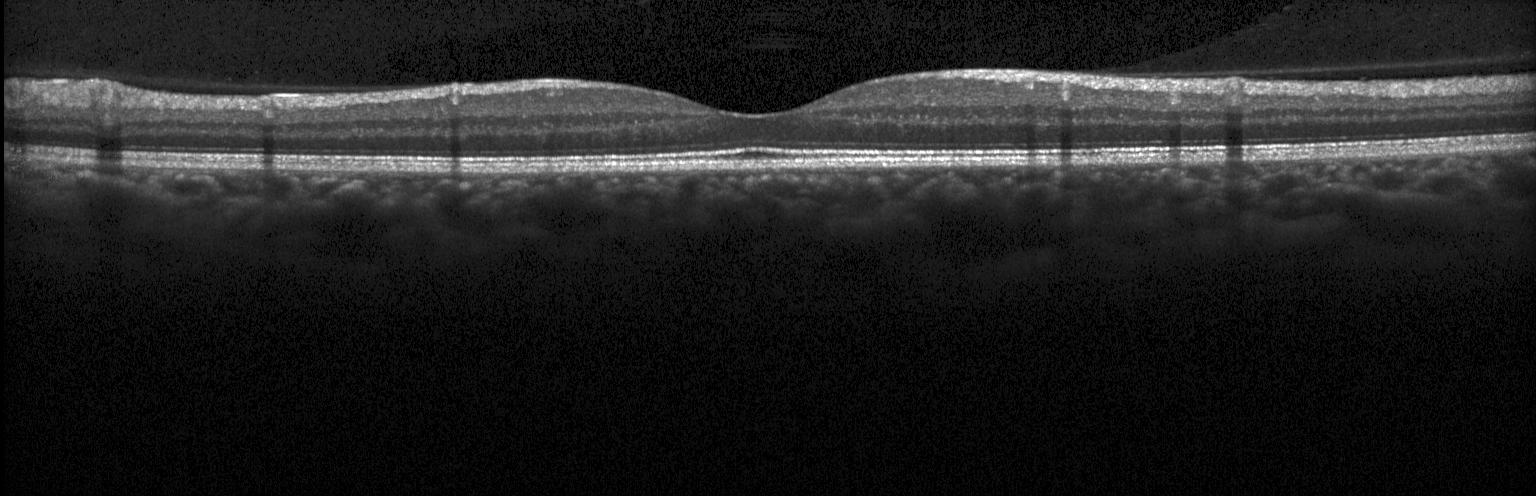
No choroidal neovascularization, no diabetic macular edema, and no drusen.